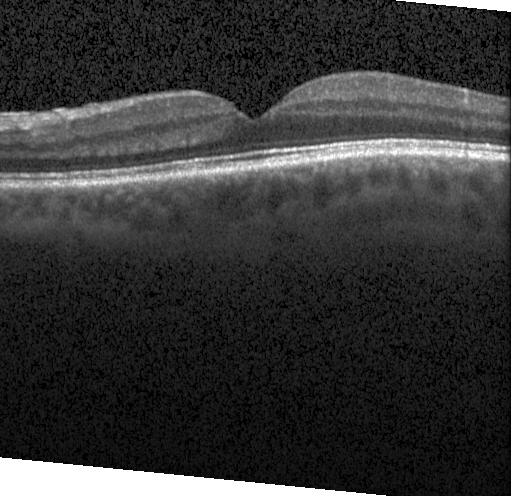

Centered on the fovea. SD-OCT. OCT line scan. Heidelberg Spectralis OCT system. Impression: neither choroidal neovascularization, diabetic macular edema, nor drusen.